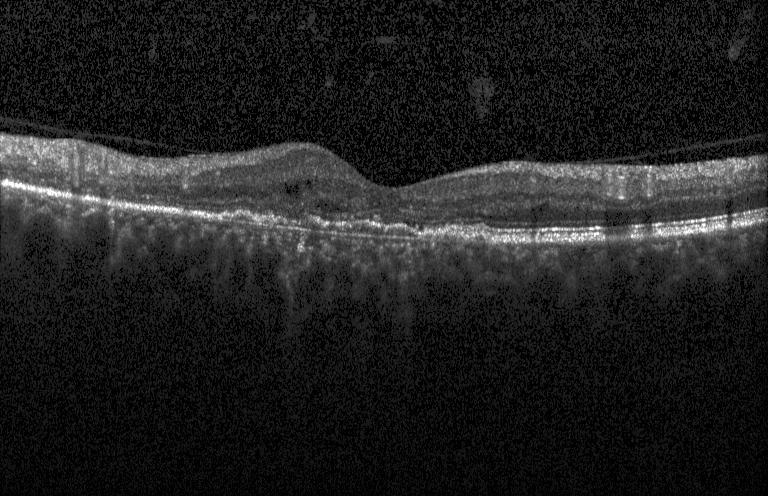
Spectral-domain OCT B-scan: choroidal neovascularization (CNV).